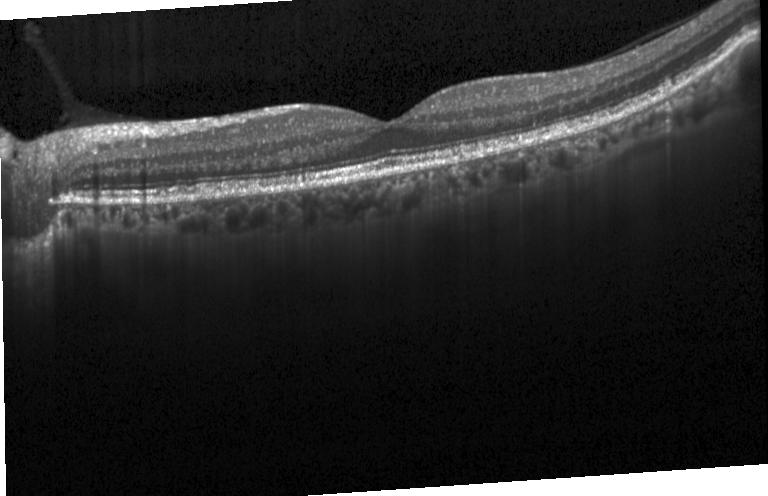 Heidelberg Spectralis OCT system · spectral-domain OCT · OCT B-scan · through the macula.
Impression: no choroidal neovascularization, no diabetic macular edema, and no drusen.